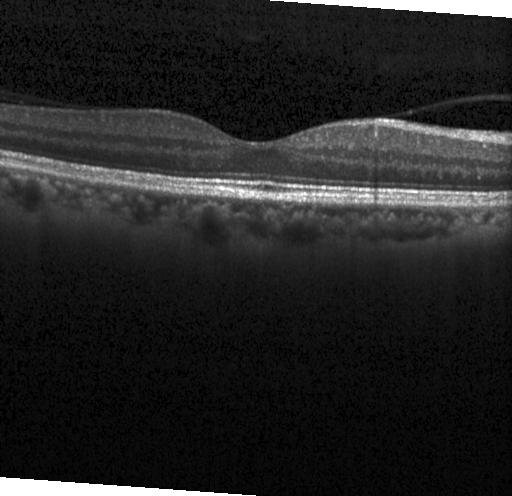 The scan shows no choroidal neovascularization, no diabetic macular edema, and no drusen.